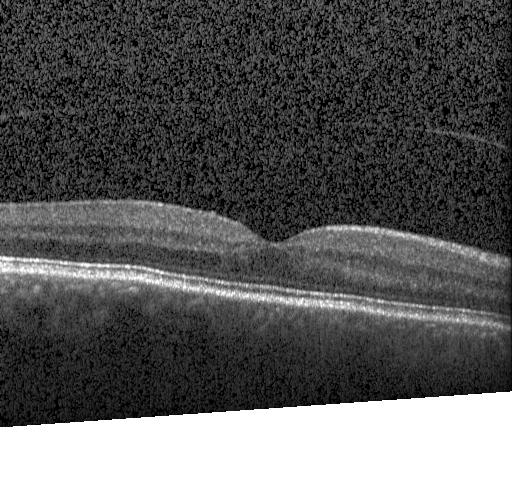

OCT B-scan.
OCT finding: no choroidal neovascularization, diabetic macular edema, or drusen.